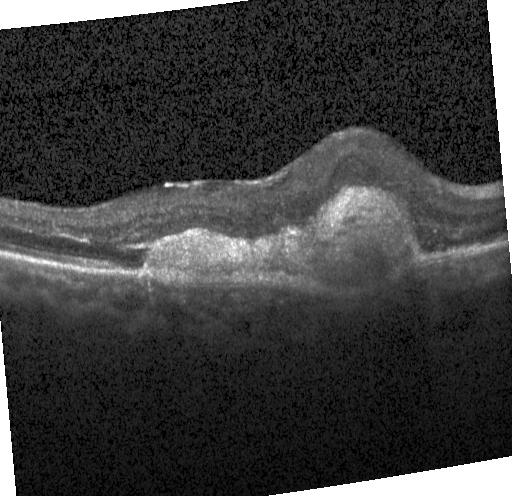

OCT B-scan showing choroidal neovascularization (CNV).